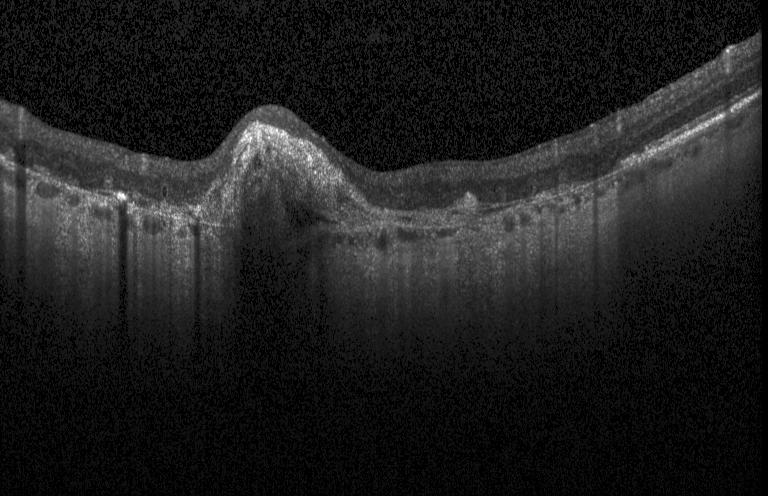 Heidelberg Spectralis, SD-OCT, optical coherence tomography B-scan, macular scan
Impression: a choroidal neovascular membrane.